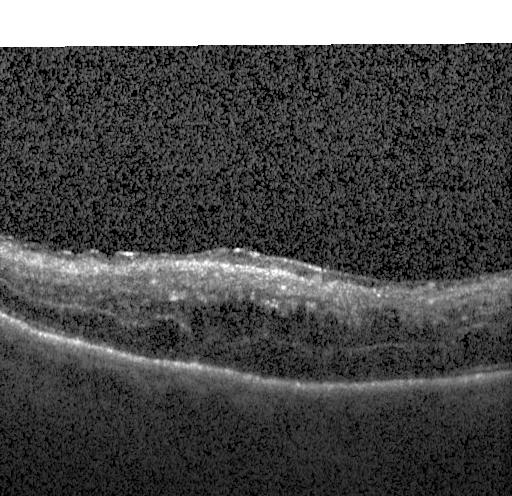
Optical coherence tomography B-scan · macular scan
This B-scan demonstrates diabetic macular edema.